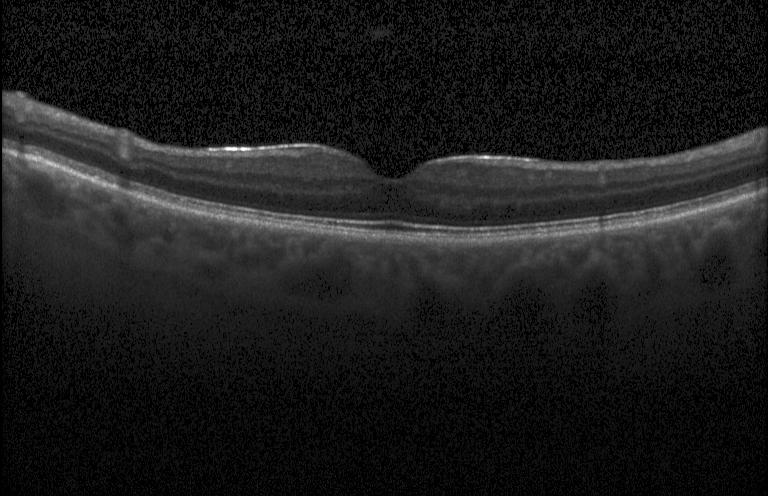
Spectral-domain optical coherence tomography; fovea-centered; retinal OCT cross-section; Heidelberg Spectralis. Finding: no choroidal neovascularization, diabetic macular edema, or drusen.